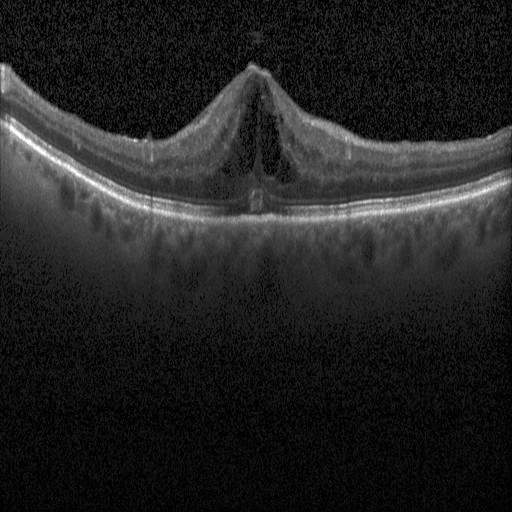
Assessment: diabetic macular edema (DME).